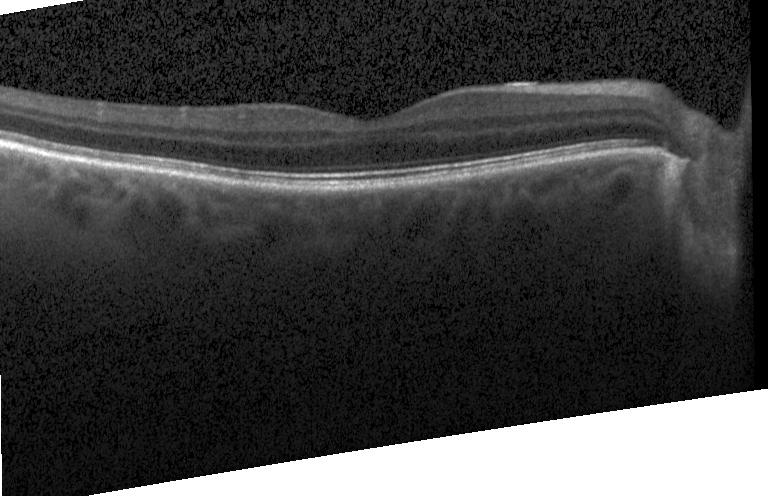

Impression: no evidence of choroidal neovascularization, diabetic macular edema, or drusen.